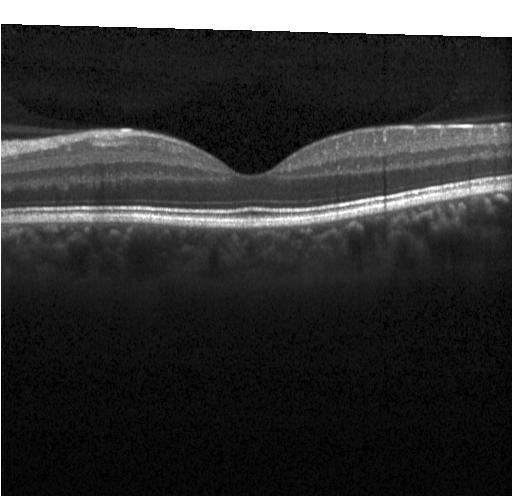 Macular OCT: no choroidal neovascularization, no diabetic macular edema, and no drusen.